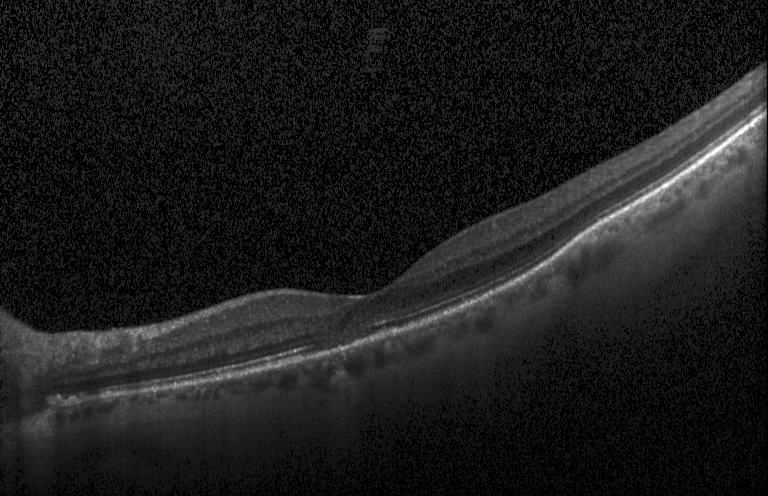 Instrument: Heidelberg Spectralis, OCT line scan, spectral-domain OCT, horizontal scan through the fovea.
Diagnosis: no CNV, DME, or drusen.